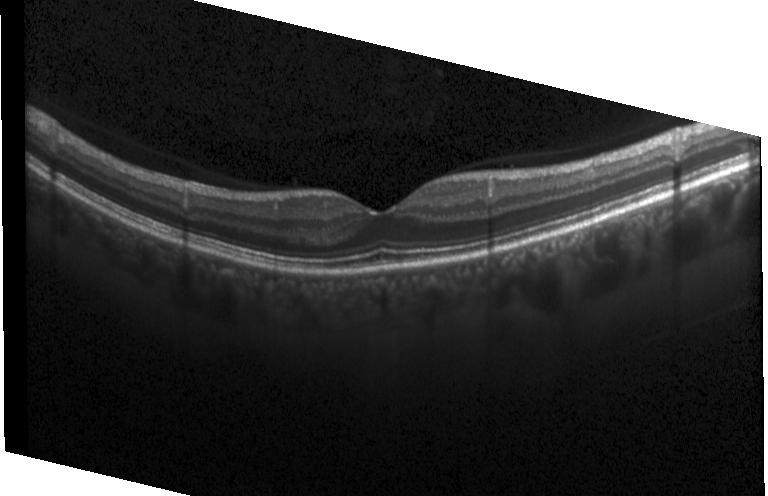

OCT B-scan. Macular scan. Heidelberg Spectralis. SD-OCT — Finding: no choroidal neovascularization, no diabetic macular edema, and no drusen.